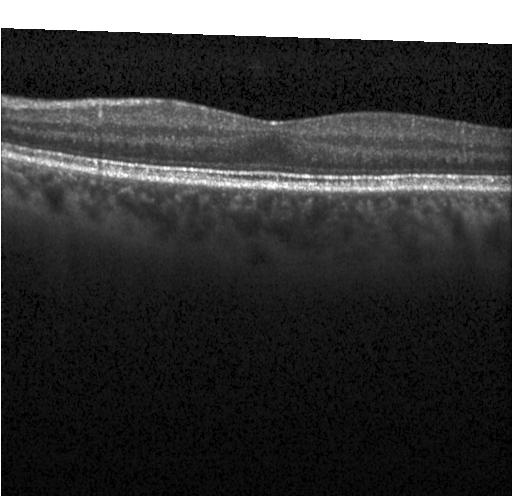 Heidelberg Spectralis, optical coherence tomography scan — OCT finding: no evidence of choroidal neovascularization, diabetic macular edema, or drusen.